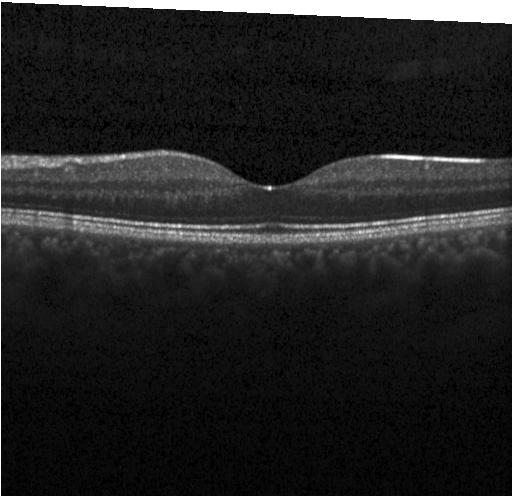 Retinal OCT cross-section showing no evidence of choroidal neovascularization, diabetic macular edema, or drusen.